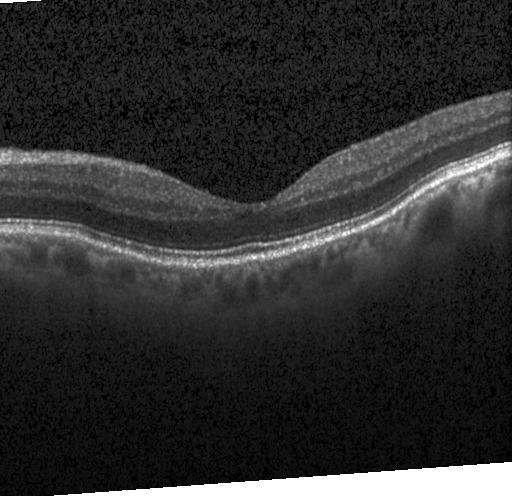

Macular scan; instrument: Heidelberg Spectralis; spectral-domain optical coherence tomography; retinal OCT B-scan — This B-scan demonstrates no evidence of CNV, DME, or drusen.